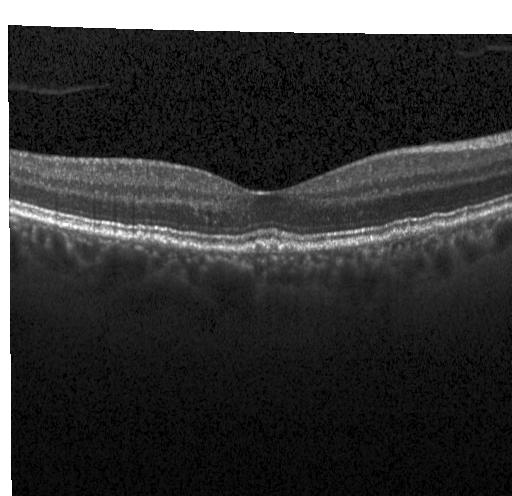 SD-OCT · OCT line scan. The scan shows drusen.